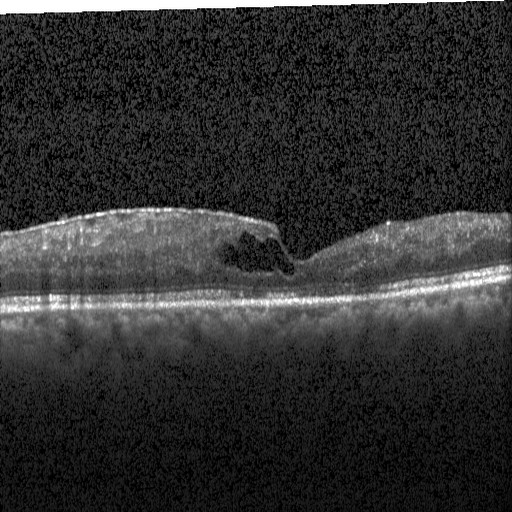 Retinal OCT B-scan
The scan shows diabetic macular edema.